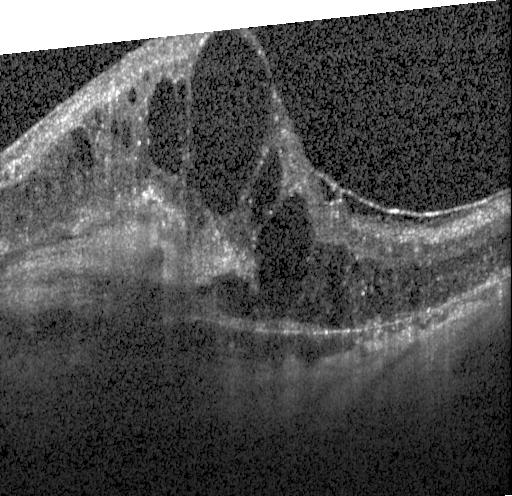

Fovea-centered. Retinal OCT cross-section.
Diagnosis: choroidal neovascularization (CNV).